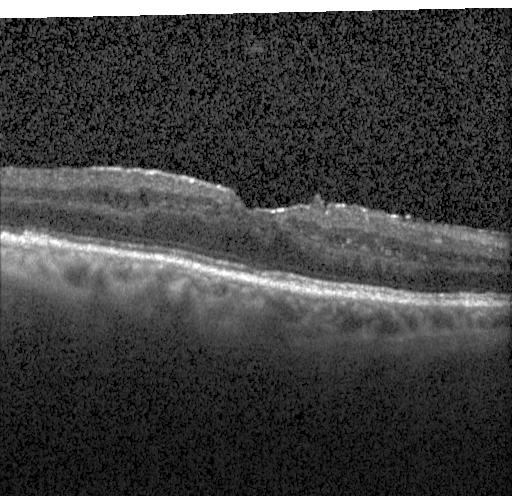

Diagnosis: DME.